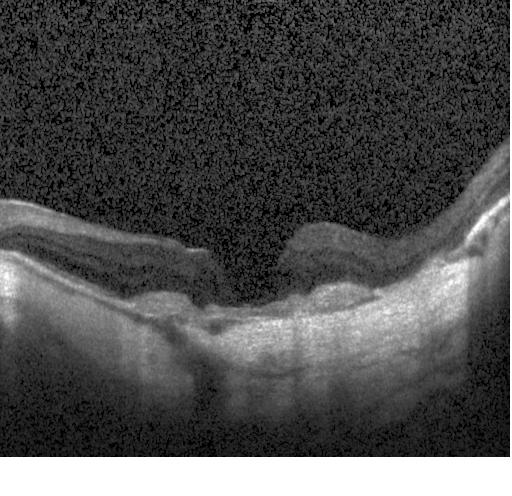 Macular OCT demonstrating choroidal neovascularization.